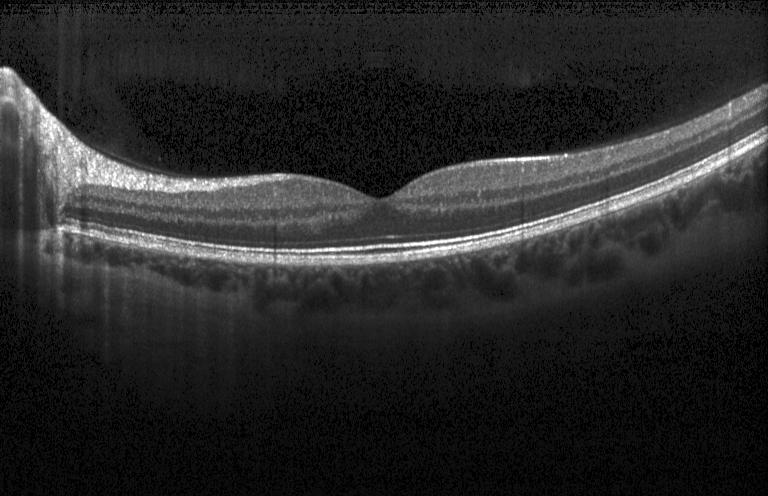 Spectral-domain OCT B-scan: neither choroidal neovascularization, diabetic macular edema, nor drusen.